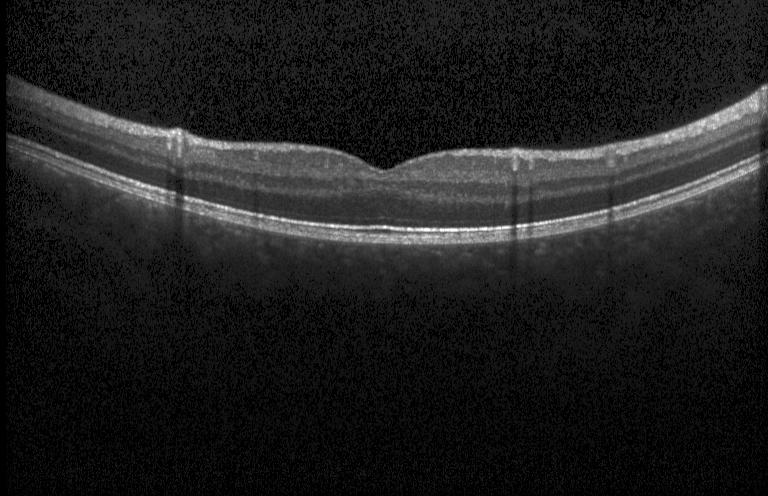

Retinal OCT B-scan; spectral-domain optical coherence tomography.
This B-scan demonstrates no evidence of choroidal neovascularization, diabetic macular edema, or drusen.